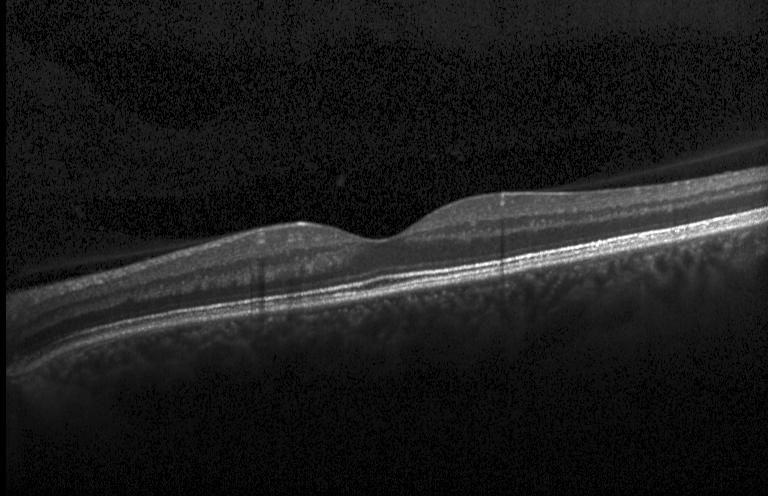

No CNV, DME, or drusen.